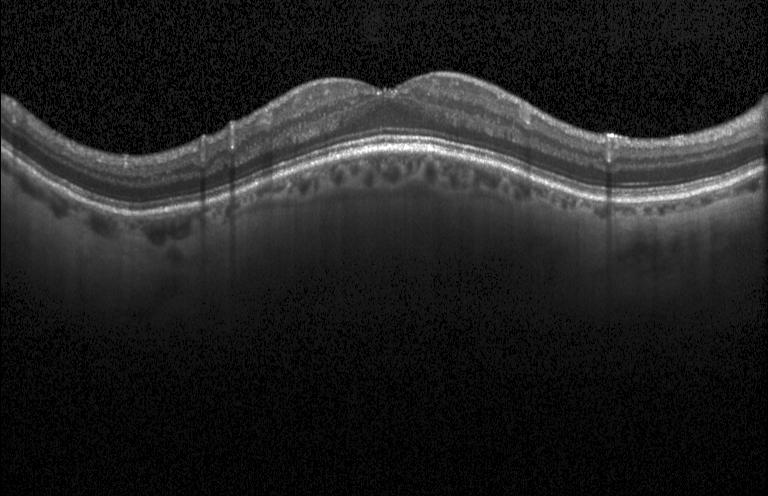
OCT line scan. Centered on the fovea. Spectral-domain OCT
Macular OCT: no choroidal neovascularization, diabetic macular edema, or drusen.